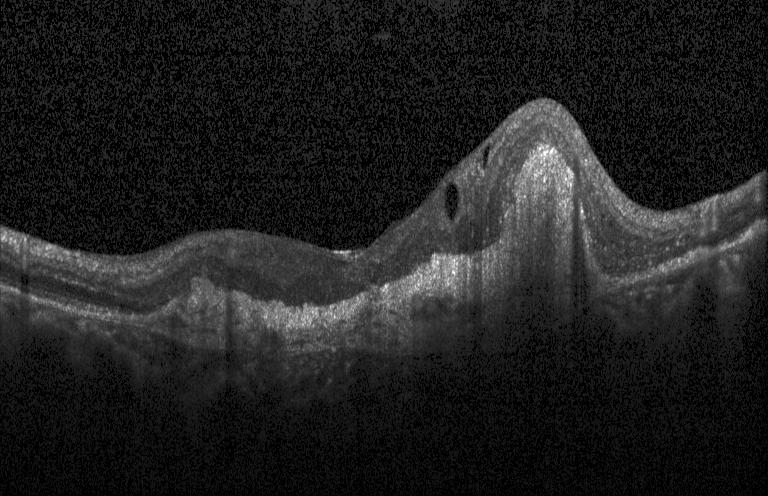
Optical coherence tomography scan; instrument: Heidelberg Spectralis; SD-OCT; macular scan. Finding: CNV.